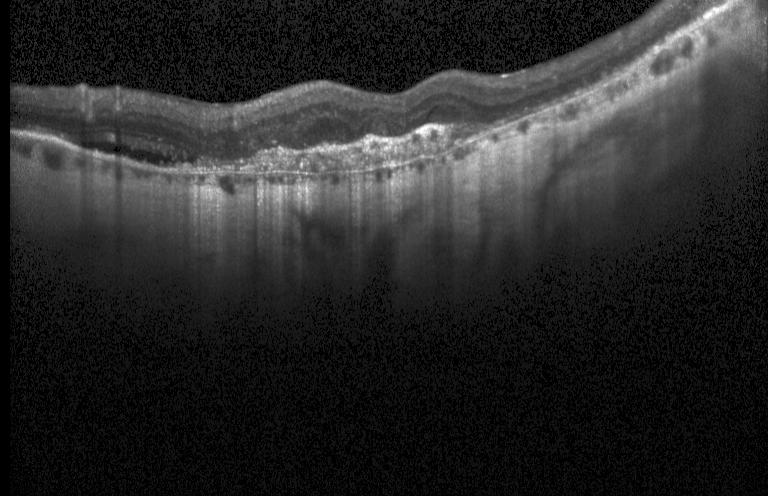

A choroidal neovascular membrane.